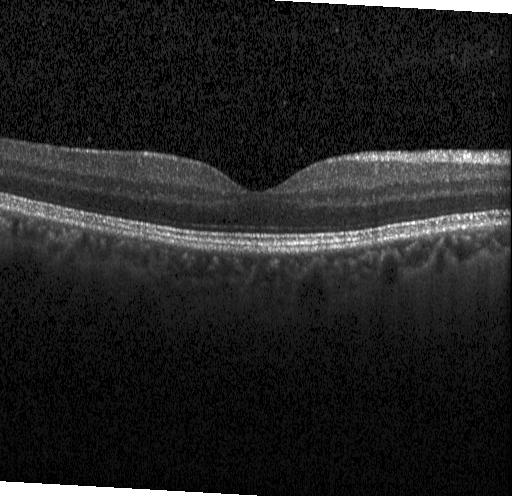

Optical coherence tomography B-scan. No choroidal neovascularization, diabetic macular edema, or drusen.